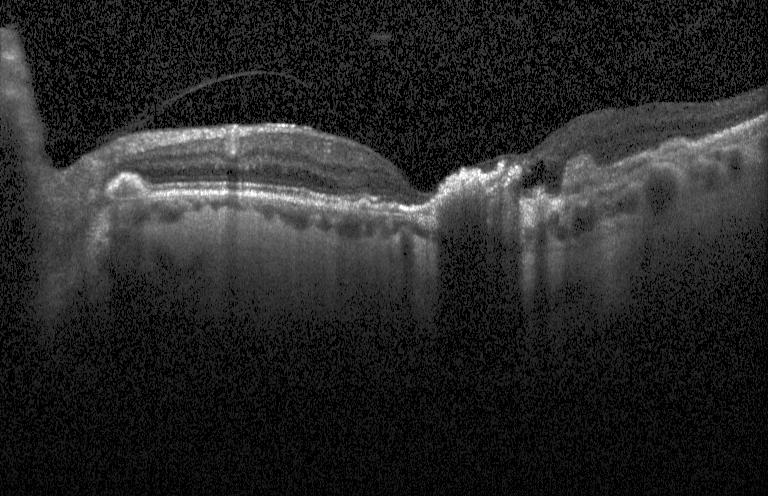 Retinal OCT B-scan, fovea-centered, acquired on a Heidelberg Spectralis.
Impression: a choroidal neovascular membrane.